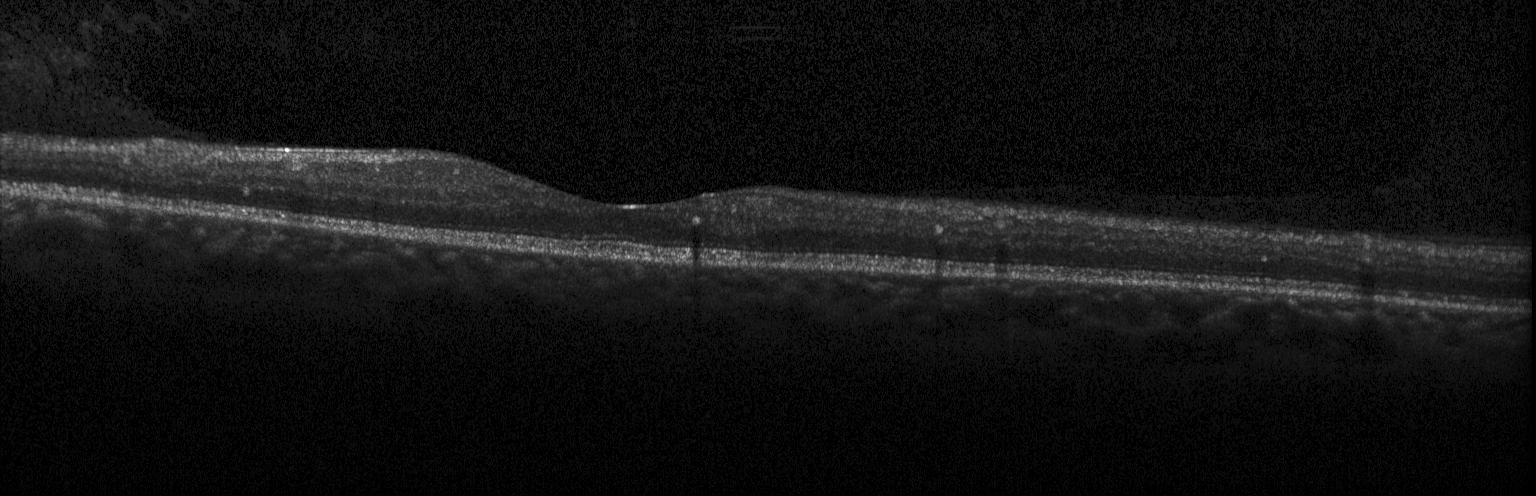

Finding: diabetic macular edema.